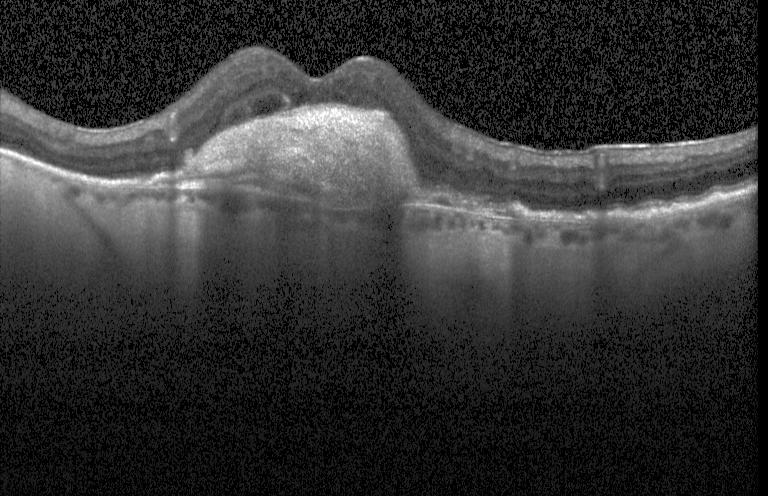
Impression: a choroidal neovascular membrane.